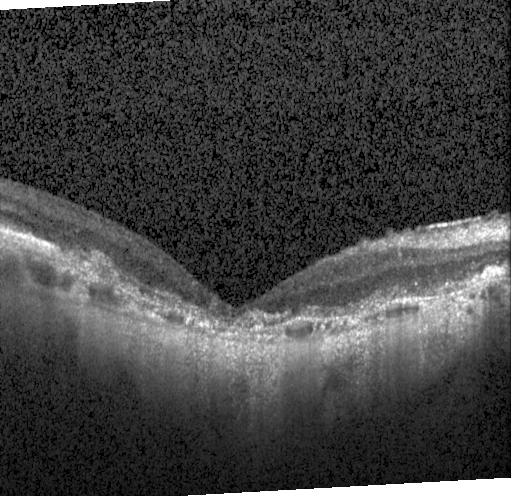

Impression: choroidal neovascularization.